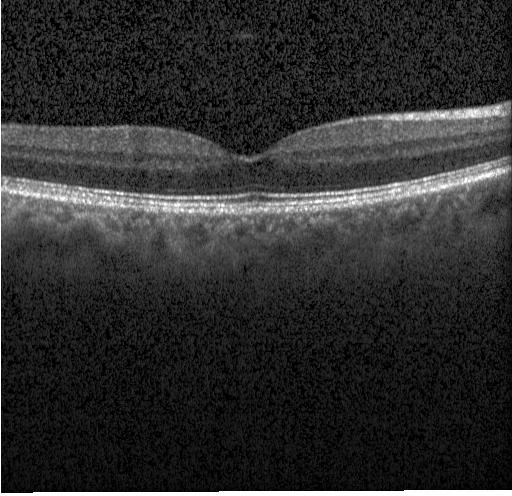
Heidelberg Spectralis, retinal OCT cross-section — Macular OCT: no CNV, no DME, and no drusen.